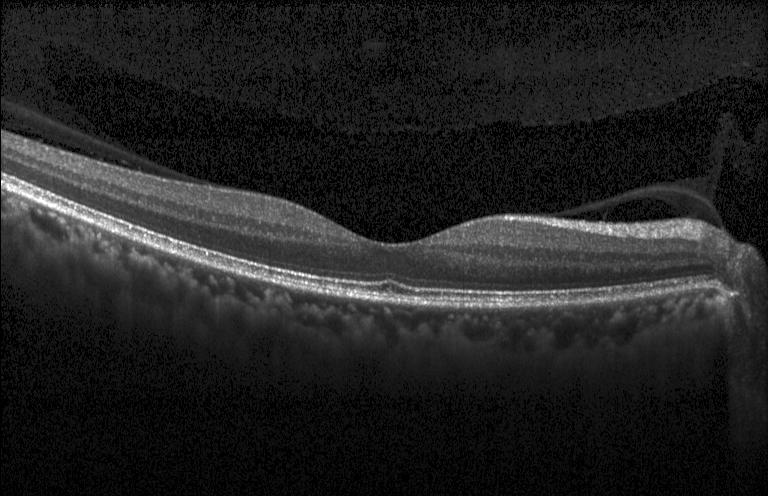
OCT B-scan, Heidelberg Spectralis, horizontal scan through the fovea, spectral-domain optical coherence tomography — Impression: no evidence of CNV, DME, or drusen.